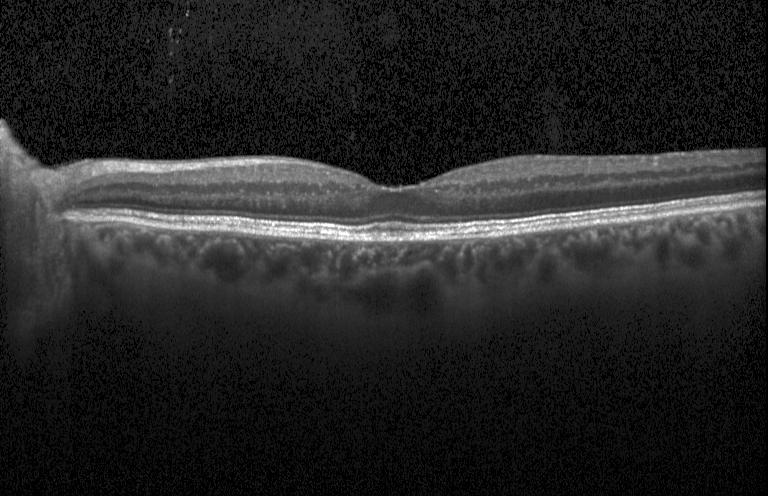 Macular OCT: no CNV, no DME, and no drusen.